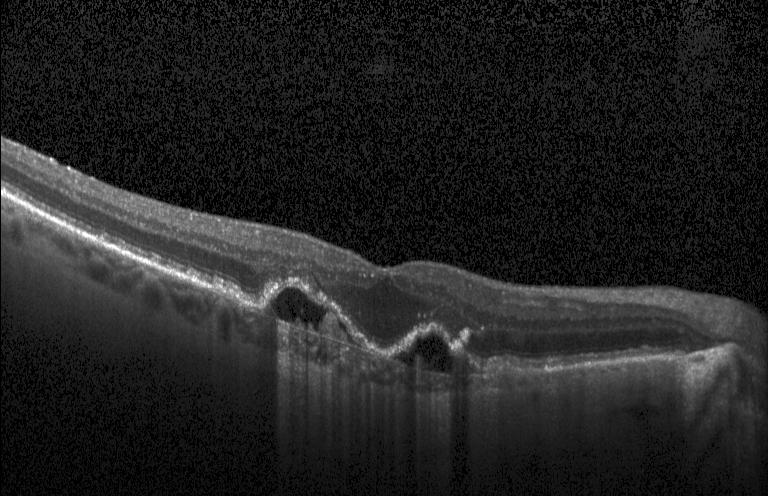
Assessment: a choroidal neovascular membrane.